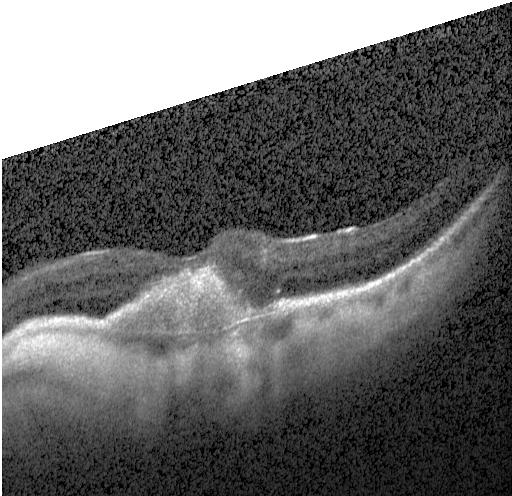

Heidelberg Spectralis · fovea-centered · optical coherence tomography scan · SD-OCT.
This B-scan demonstrates CNV.